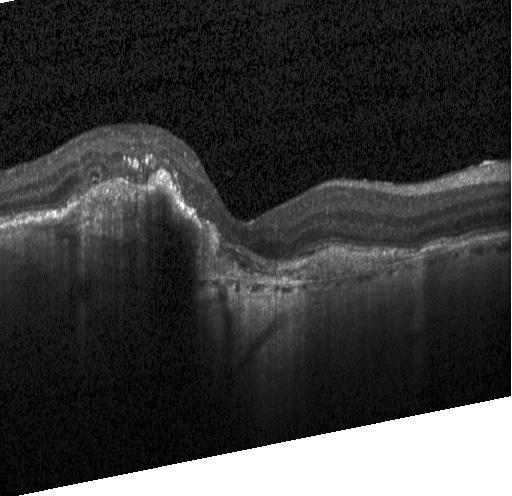
Through the macula · OCT line scan · Heidelberg Spectralis. The scan shows a choroidal neovascular membrane.